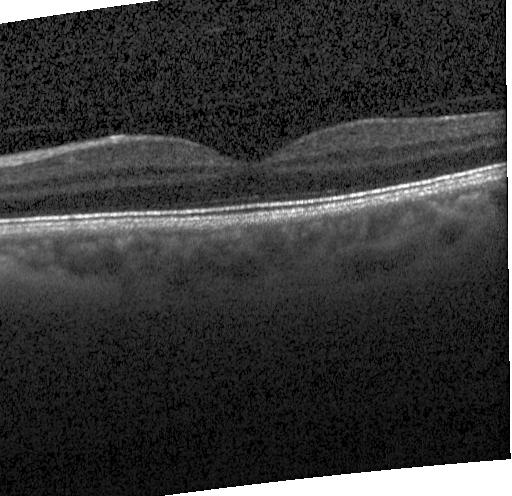
OCT finding: no choroidal neovascularization, diabetic macular edema, or drusen.